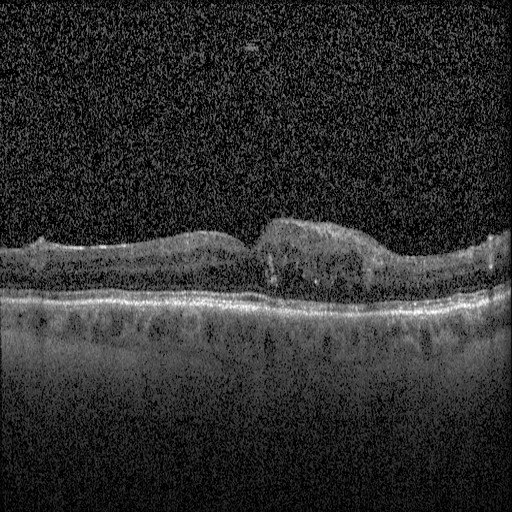
OCT B-scan; acquired on a Heidelberg Spectralis; SD-OCT.
This B-scan demonstrates DME.